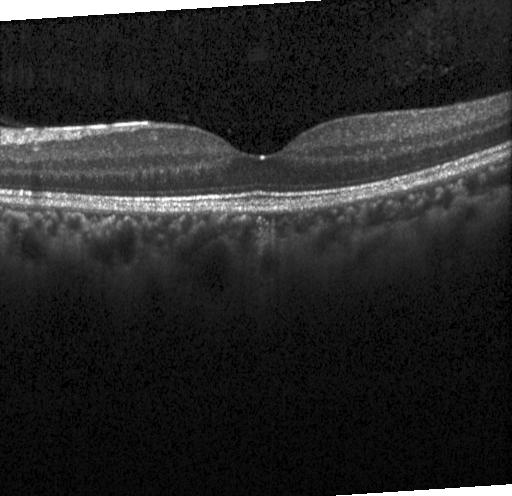
OCT B-scan. Diagnosis: neither CNV, DME, nor drusen.